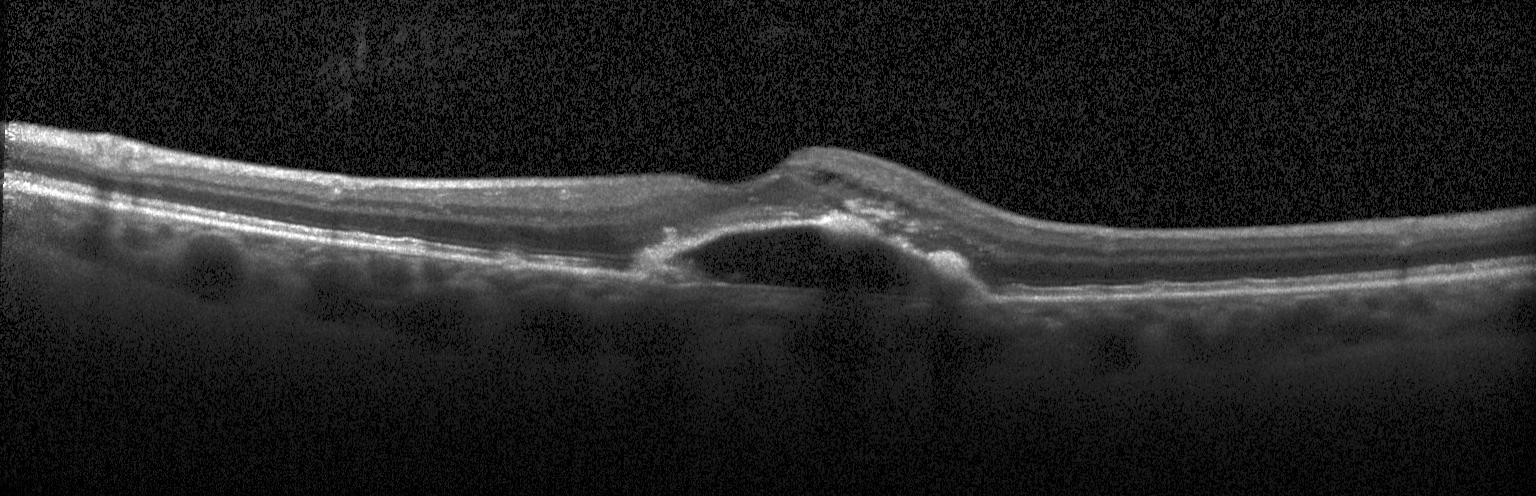 OCT scan showing choroidal neovascularization.